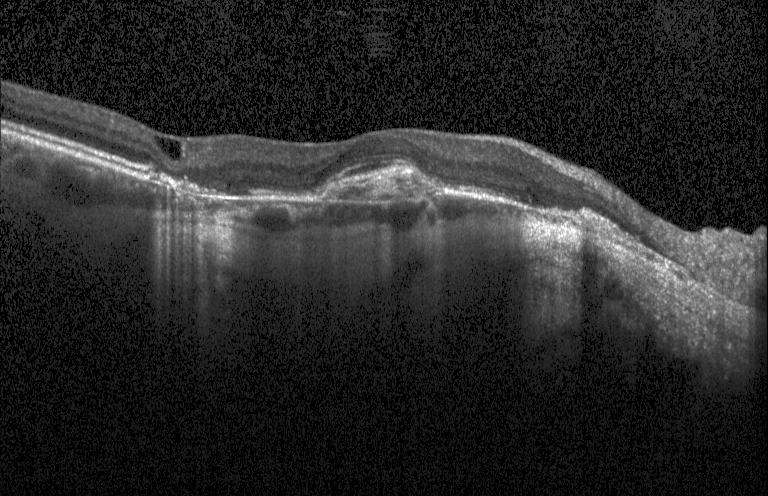

Retinal OCT cross-section — Choroidal neovascularization (CNV).